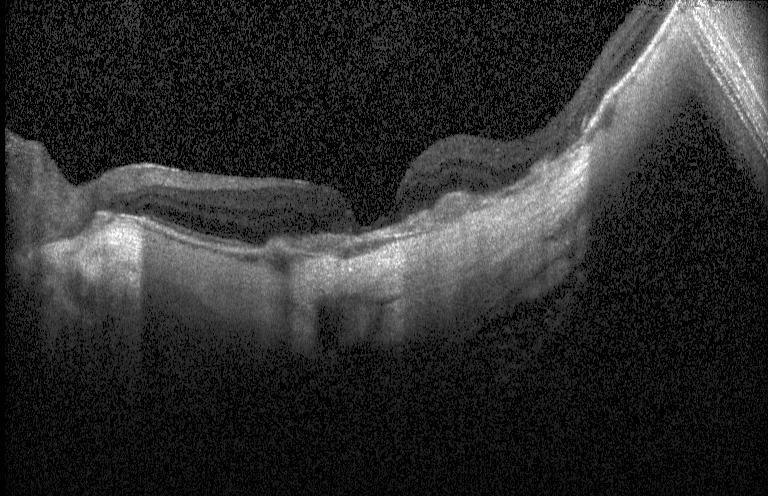
Spectral-domain optical coherence tomography · retinal OCT B-scan — Macular OCT: a choroidal neovascular membrane.